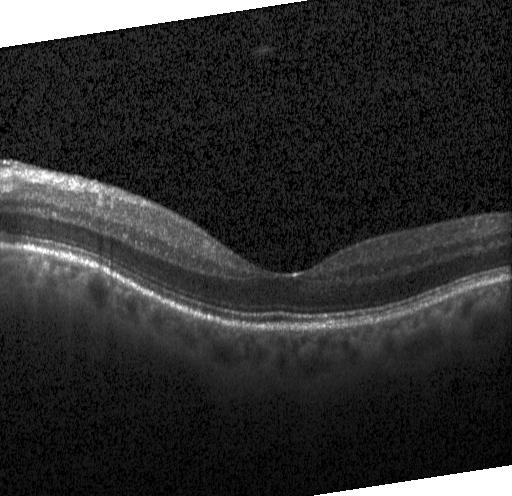

OCT line scan · horizontal scan through the fovea · SD-OCT · Heidelberg Spectralis — The scan shows neither CNV, DME, nor drusen.